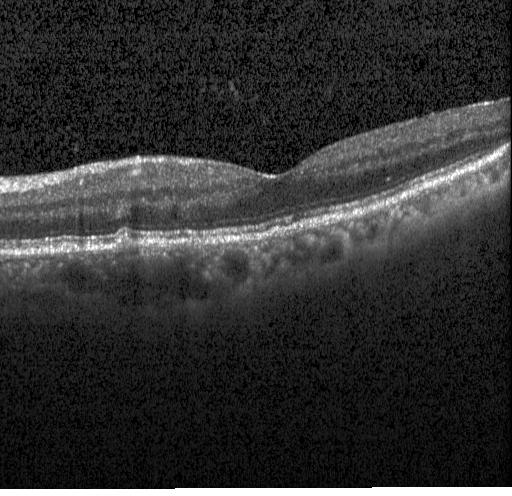
Diagnosis: multiple drusen.